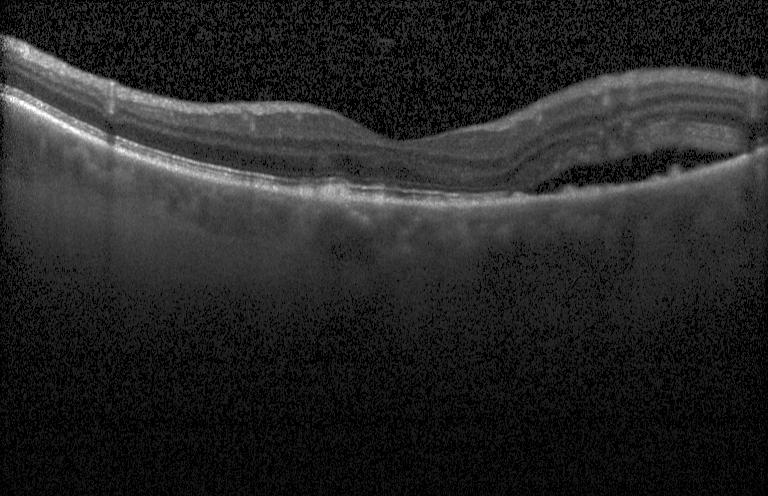
Macular OCT: choroidal neovascularization (CNV).